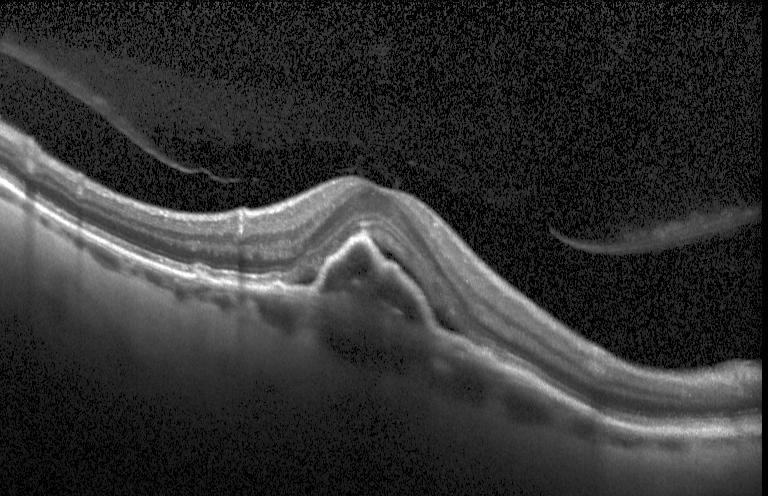
Heidelberg Spectralis, through the macula, spectral-domain optical coherence tomography, OCT B-scan. Impression: choroidal neovascularization (CNV).